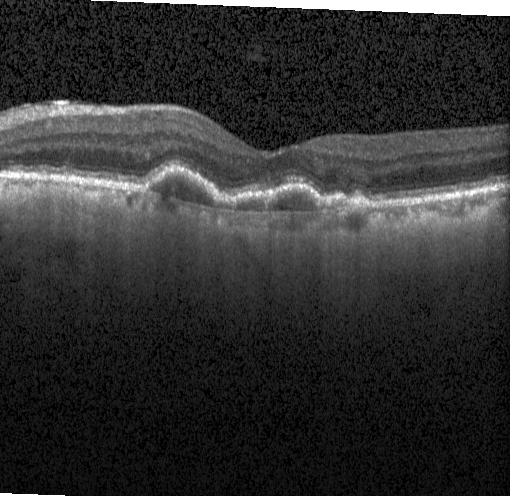

Retinal OCT cross-section.
Assessment: a choroidal neovascular membrane.